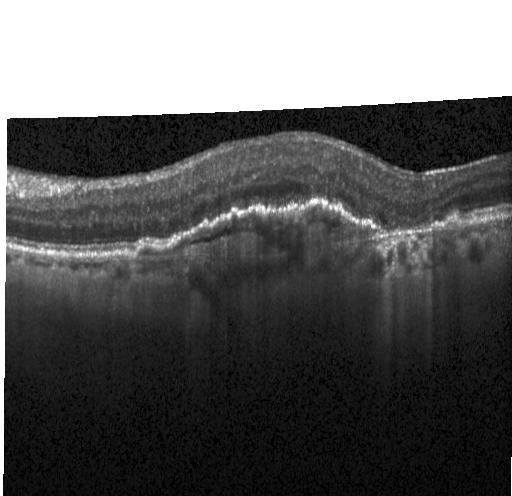 OCT finding: CNV.